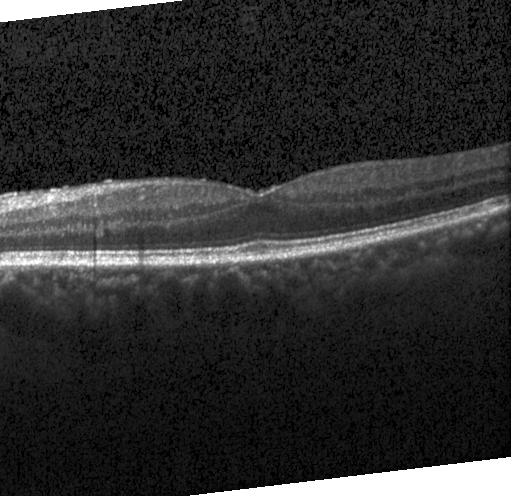 Fovea-centered · OCT B-scan.
OCT finding: no evidence of CNV, DME, or drusen.